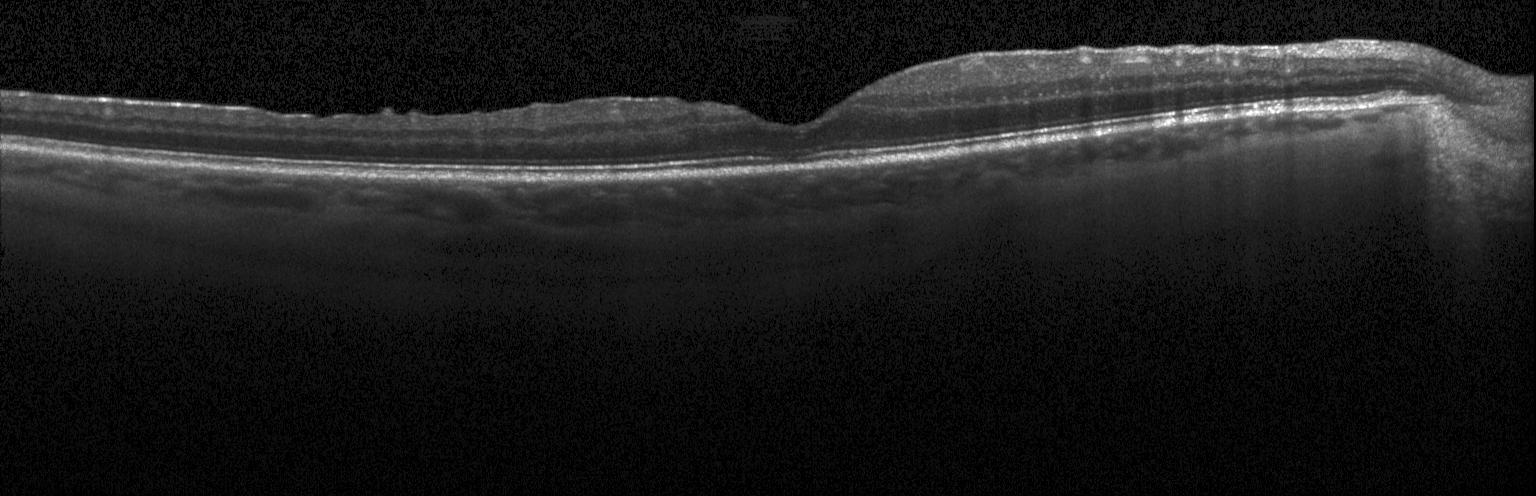

Diagnosis: no choroidal neovascularization, diabetic macular edema, or drusen.